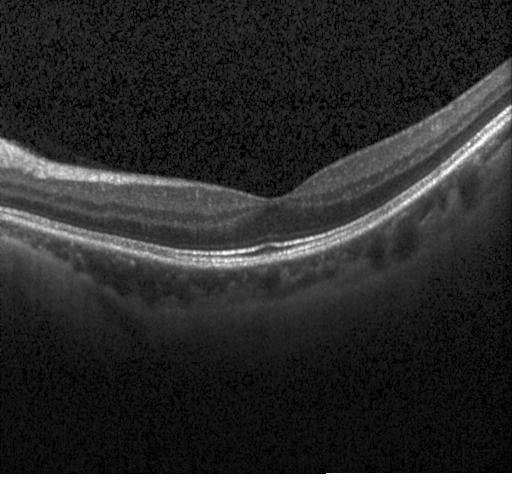 SD-OCT, acquired on a Heidelberg Spectralis, retinal OCT B-scan, fovea-centered — This B-scan demonstrates neither choroidal neovascularization, diabetic macular edema, nor drusen.